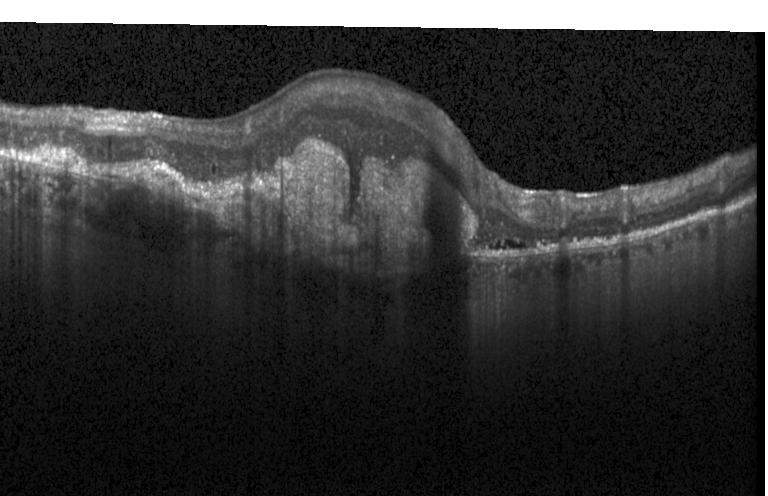
Acquired on a Heidelberg Spectralis, spectral-domain OCT, OCT B-scan, centered on the fovea — Impression: CNV.